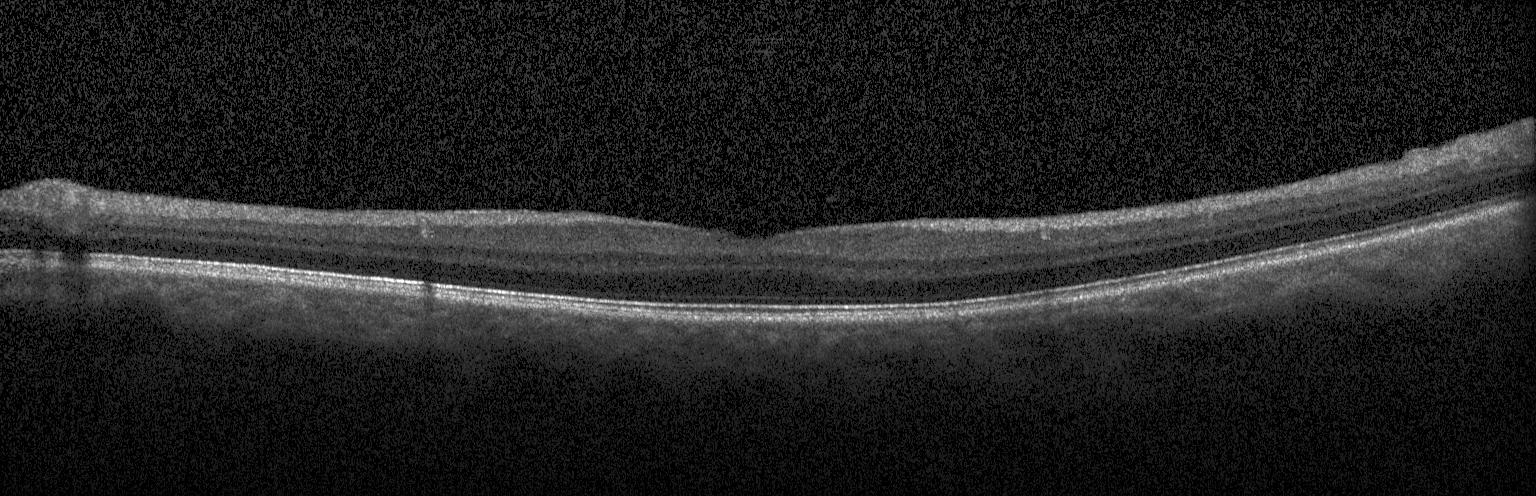
Macular scan · OCT B-scan
Impression: no choroidal neovascularization, diabetic macular edema, or drusen.